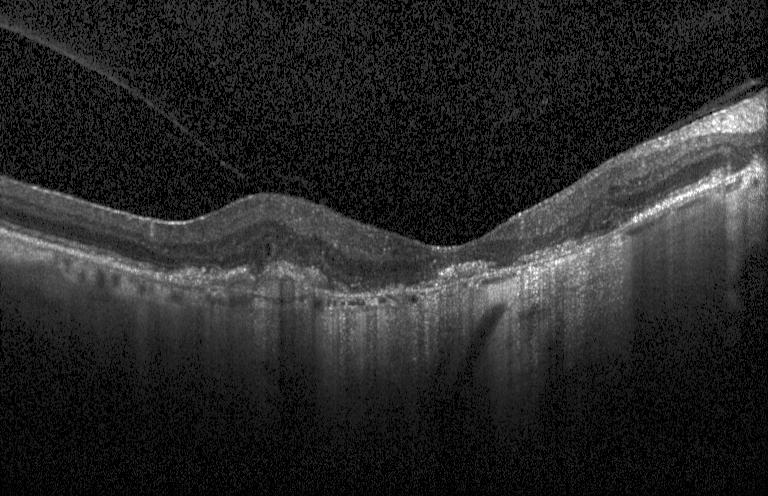

Assessment: CNV.